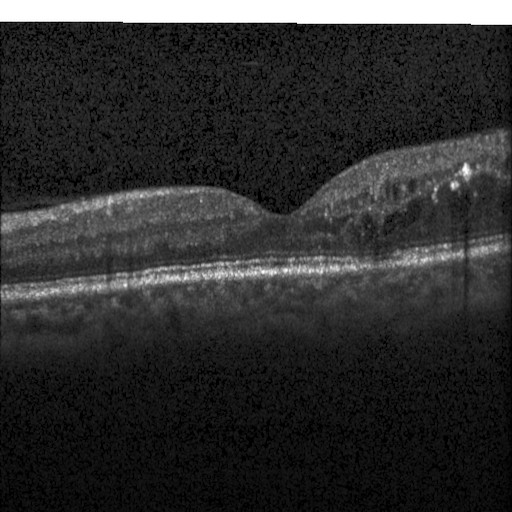 Spectral-domain OCT; OCT B-scan; through the macula — Diagnosis: diabetic macular edema (DME).